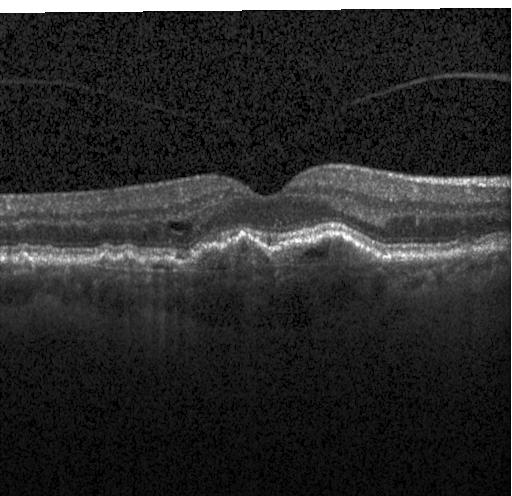
SD-OCT. Retinal OCT B-scan. Heidelberg Spectralis — Diagnosis: CNV.